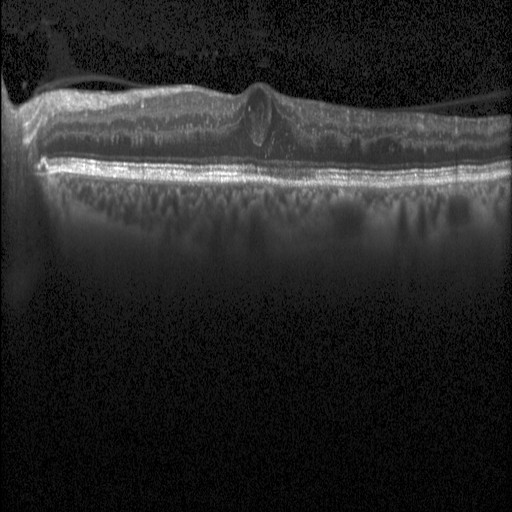 Spectral-domain OCT B-scan: diabetic macular edema (DME).